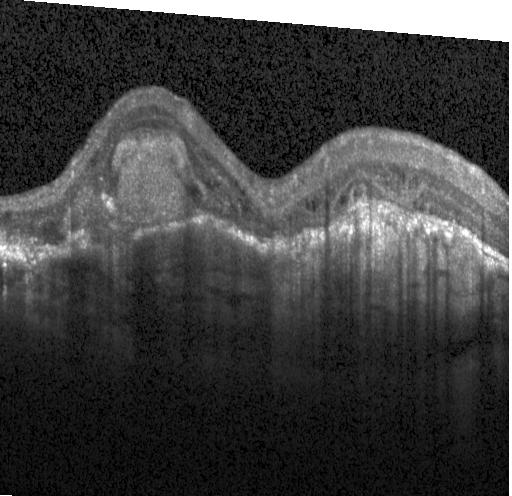 Retinal OCT cross-section. Assessment: CNV.